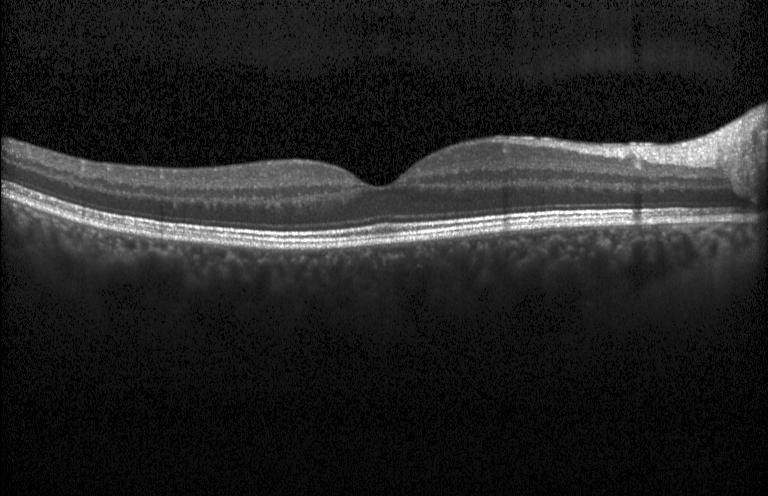

Spectral-domain optical coherence tomography; OCT line scan
OCT finding: no CNV, no DME, and no drusen.